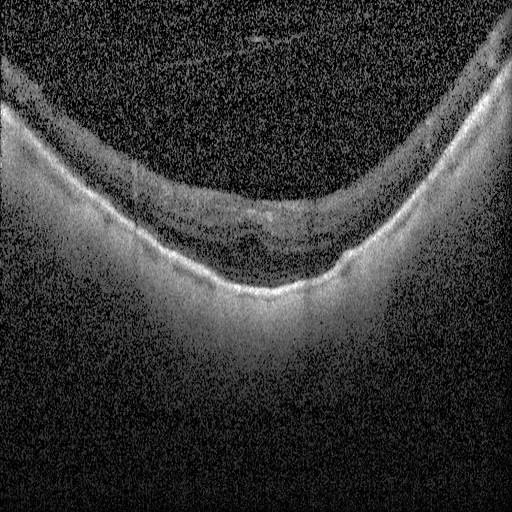
Spectral-domain OCT B-scan: DME.